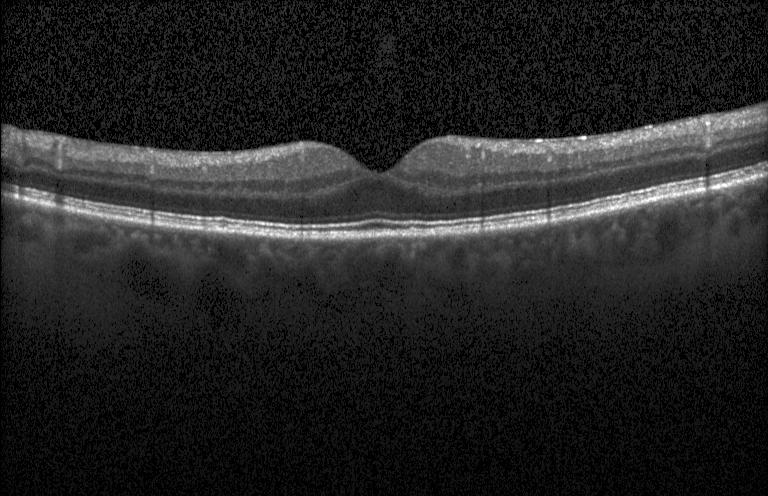
Finding: no choroidal neovascularization, diabetic macular edema, or drusen.